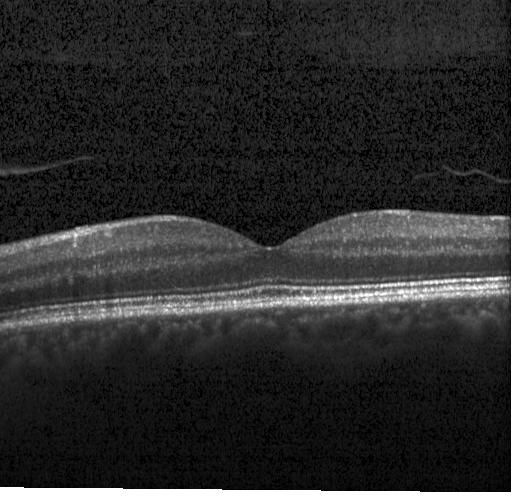 OCT B-scan, instrument: Heidelberg Spectralis. This B-scan demonstrates neither CNV, DME, nor drusen.